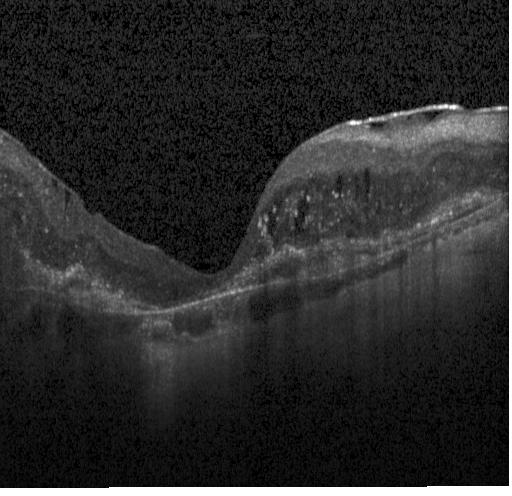
Finding: a choroidal neovascular membrane.